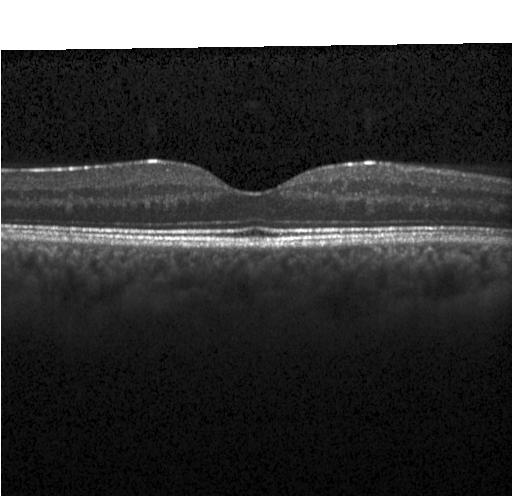

SD-OCT; optical coherence tomography B-scan.
No CNV, DME, or drusen.